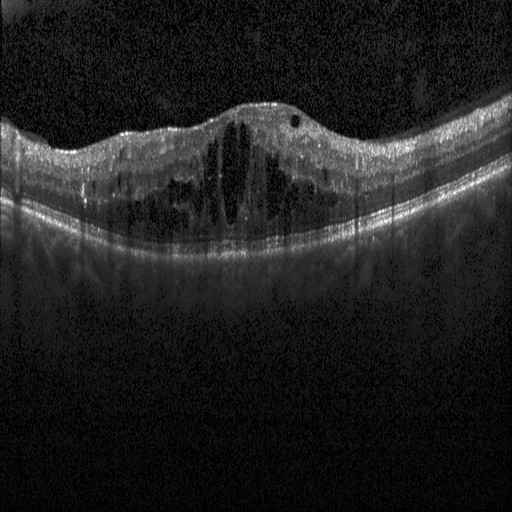

Finding: diabetic macular edema (DME).